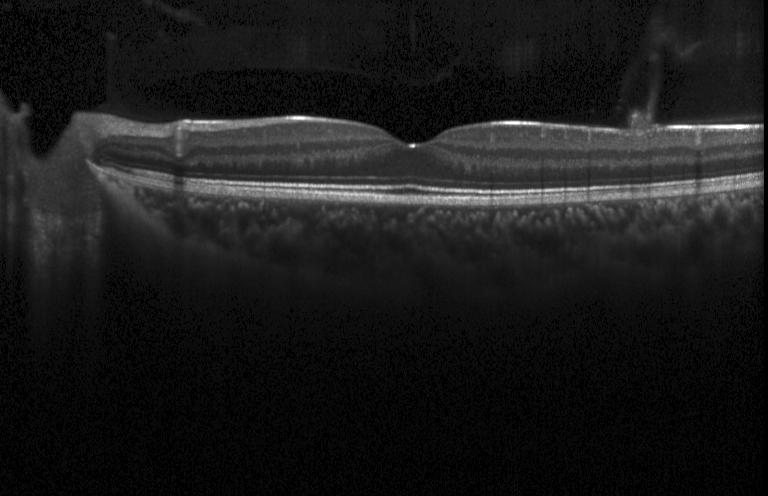 OCT B-scan showing no choroidal neovascularization, diabetic macular edema, or drusen.